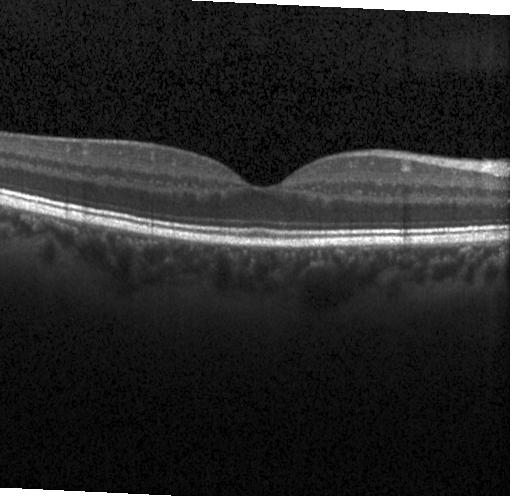

Spectral-domain OCT B-scan: no evidence of choroidal neovascularization, diabetic macular edema, or drusen.